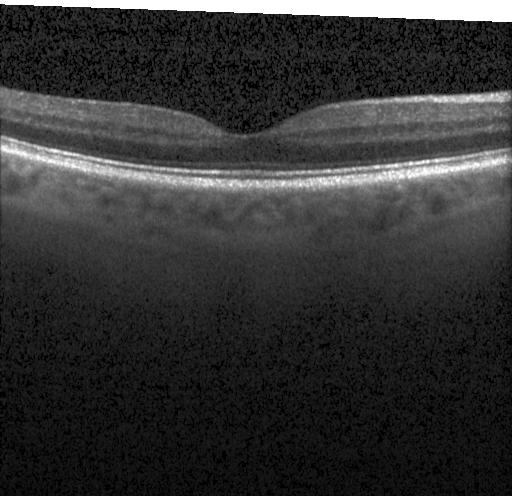
Finding: no evidence of CNV, DME, or drusen.